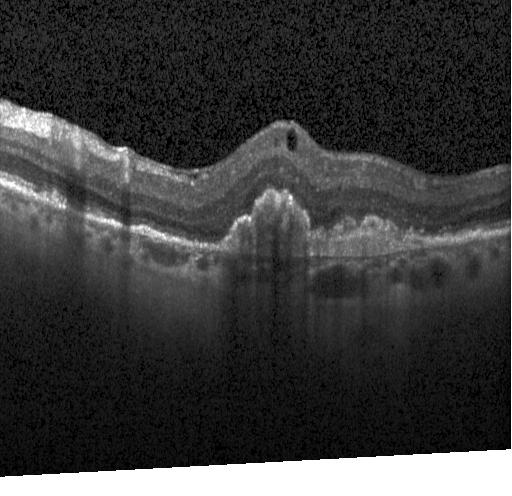 Acquired on a Heidelberg Spectralis; fovea-centered; optical coherence tomography scan; spectral-domain OCT — Assessment: choroidal neovascularization.